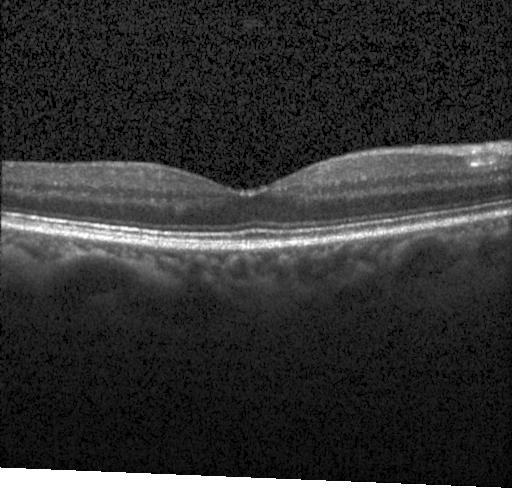 Acquired on a Heidelberg Spectralis, spectral-domain OCT, centered on the fovea, retinal OCT B-scan
Finding: no choroidal neovascularization, no diabetic macular edema, and no drusen.